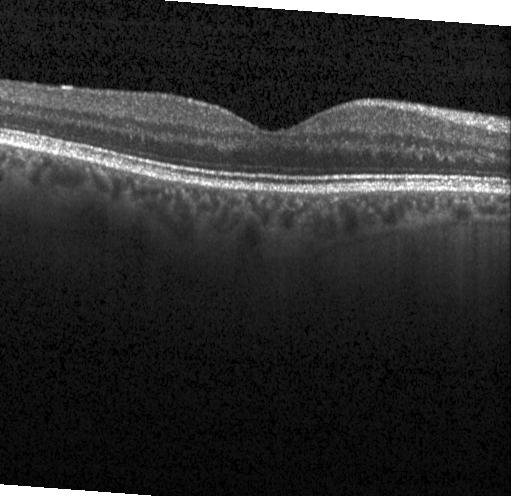 Retinal OCT B-scan, spectral-domain OCT. Impression: no CNV, no DME, and no drusen.